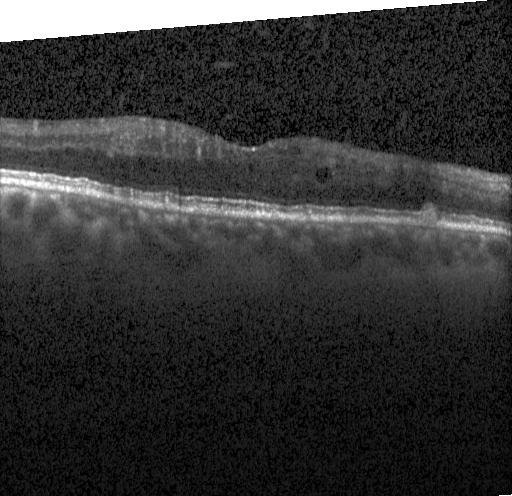

Impression: DME.